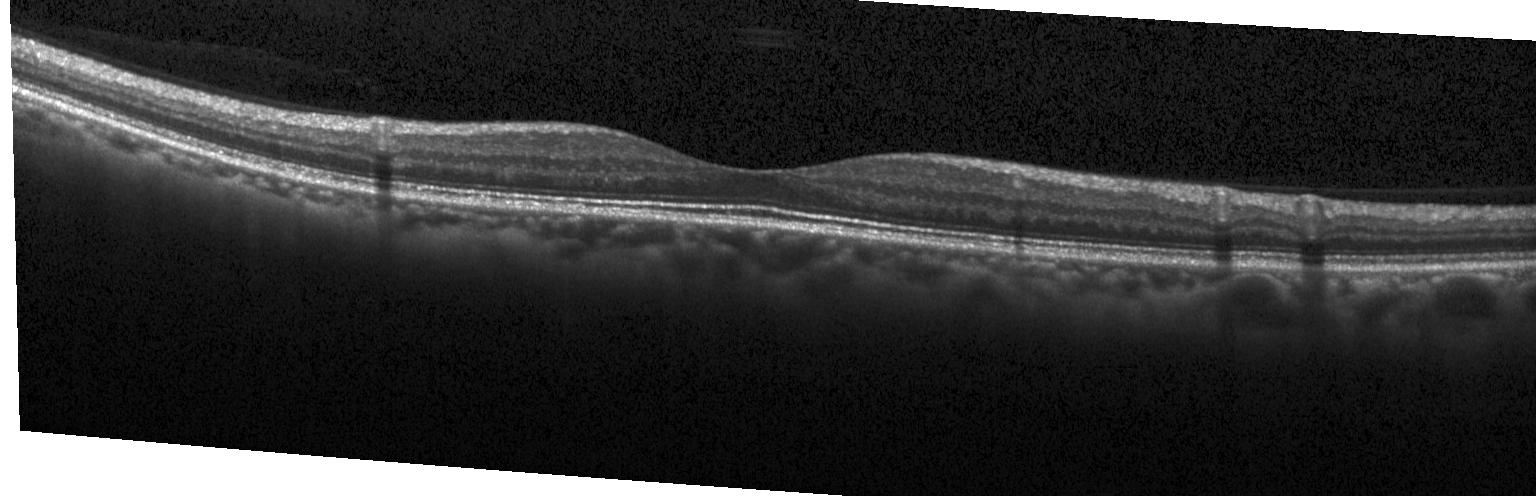
Optical coherence tomography scan, instrument: Heidelberg Spectralis, centered on the fovea. Diagnosis: no choroidal neovascularization, no diabetic macular edema, and no drusen.